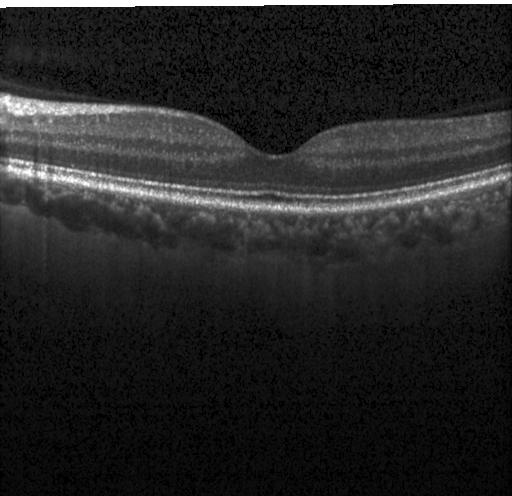 Retinal OCT B-scan — Diagnosis: no CNV, no DME, and no drusen.